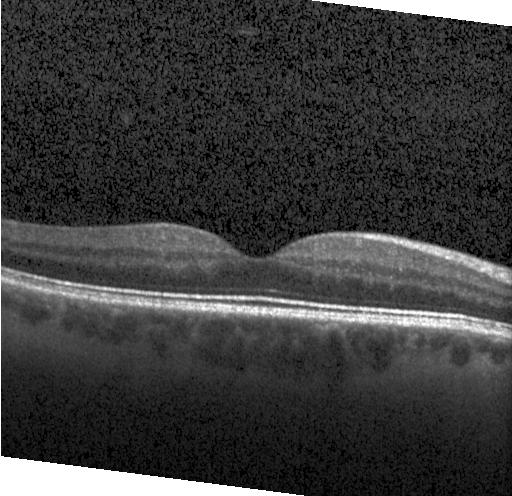

Diagnosis: no CNV, DME, or drusen.